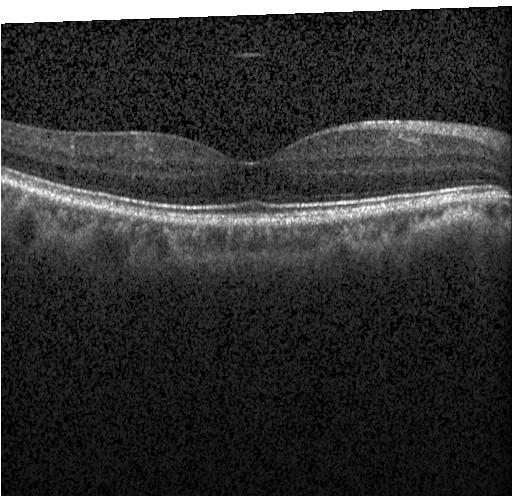
Retinal OCT cross-section showing no evidence of choroidal neovascularization, diabetic macular edema, or drusen.